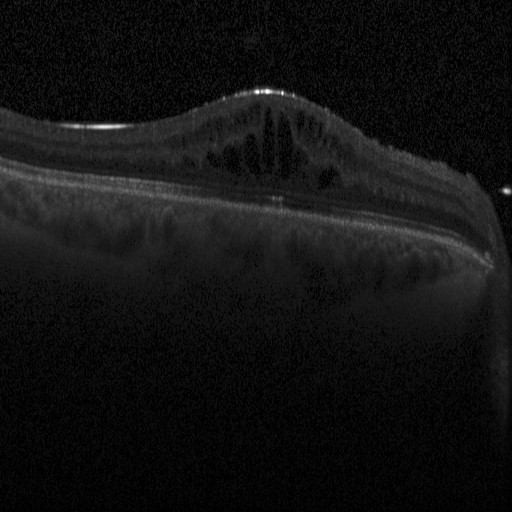

Impression: diabetic macular edema (DME).